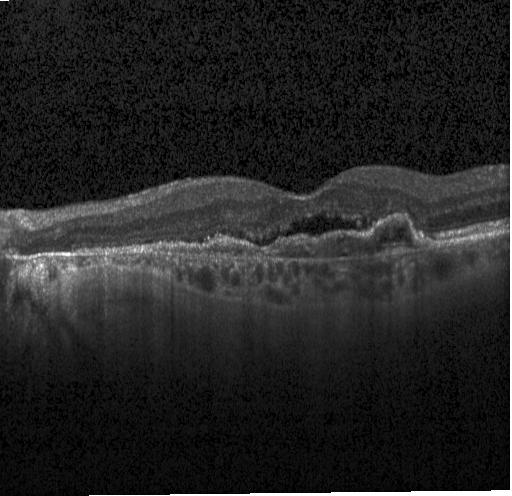
Diagnosis: choroidal neovascularization (CNV).